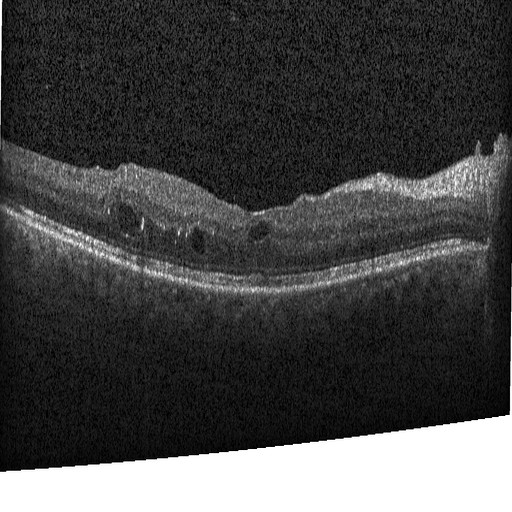

Finding: diabetic macular edema (DME).